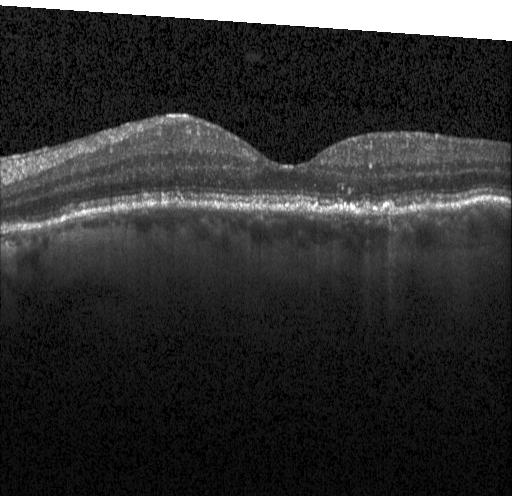
OCT B-scan showing drusen.